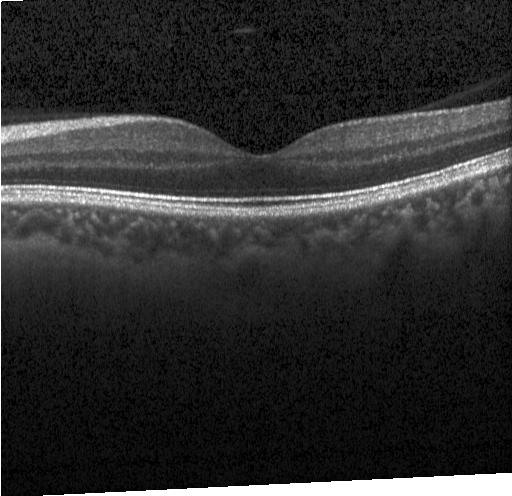
Heidelberg Spectralis, retinal OCT B-scan.
No choroidal neovascularization, no diabetic macular edema, and no drusen.